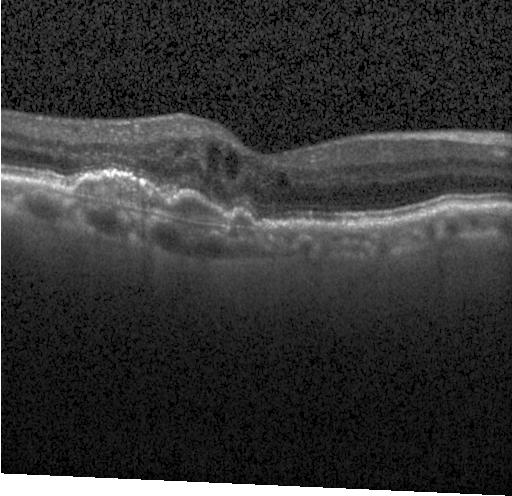

OCT line scan, spectral-domain optical coherence tomography. Choroidal neovascularization.